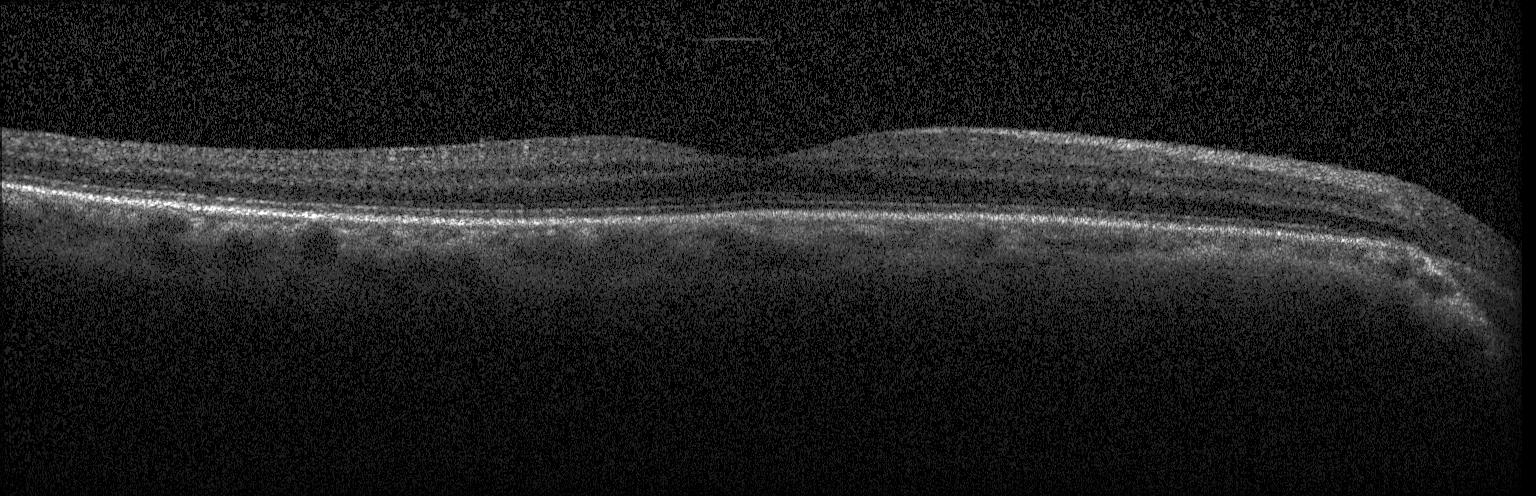

Retinal OCT cross-section
Impression: no evidence of choroidal neovascularization, diabetic macular edema, or drusen.